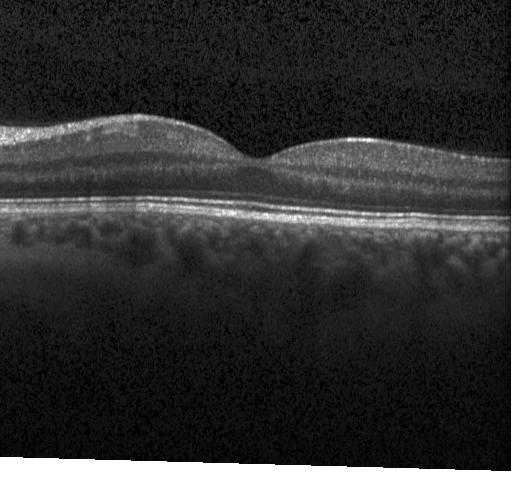
Finding: neither choroidal neovascularization, diabetic macular edema, nor drusen.